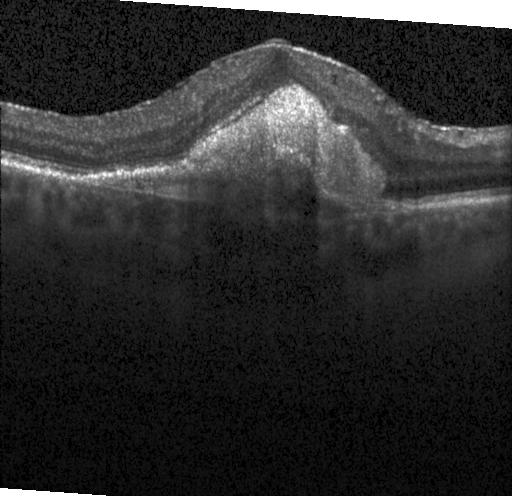
Retinal OCT cross-section; acquired on a Heidelberg Spectralis; spectral-domain optical coherence tomography
Impression: choroidal neovascularization.